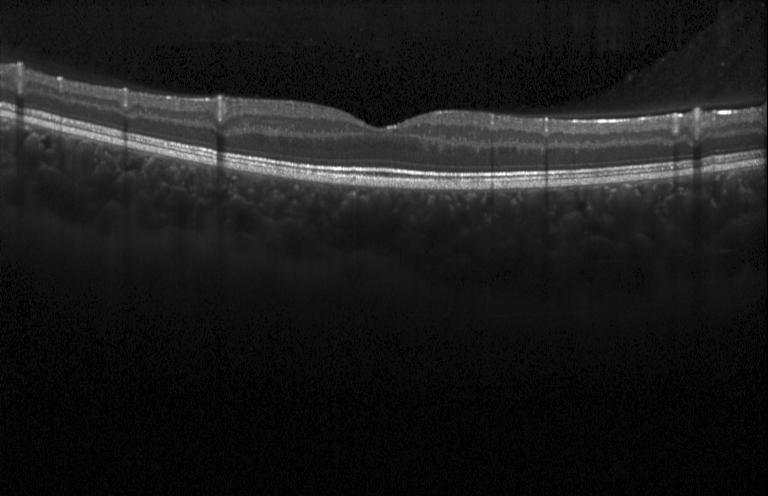
Dx: no CNV, DME, or drusen.